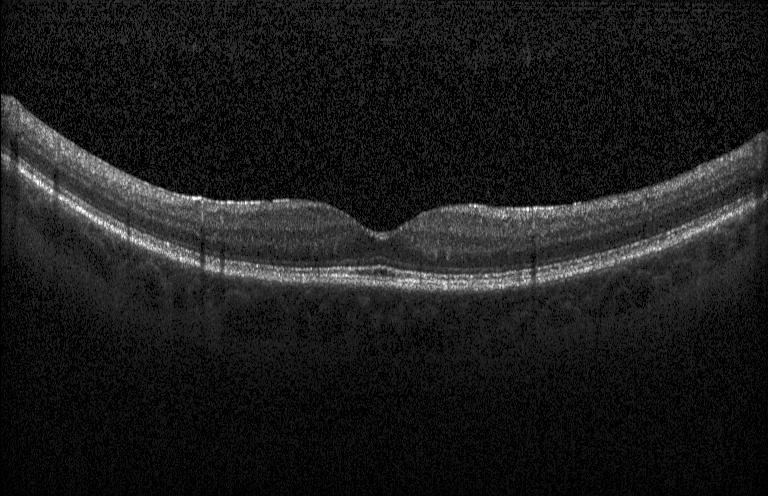 Retinal OCT cross-section showing no CNV, DME, or drusen.